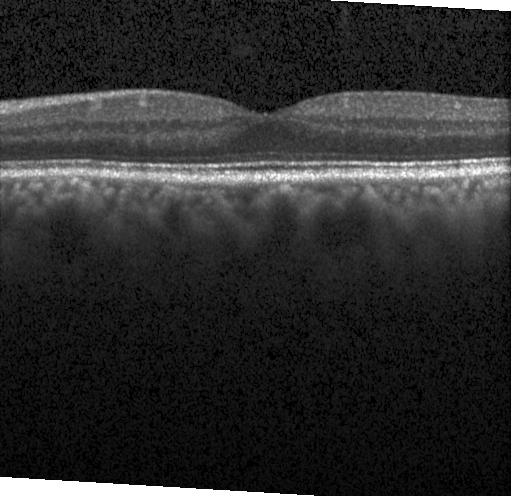 Finding: neither choroidal neovascularization, diabetic macular edema, nor drusen.